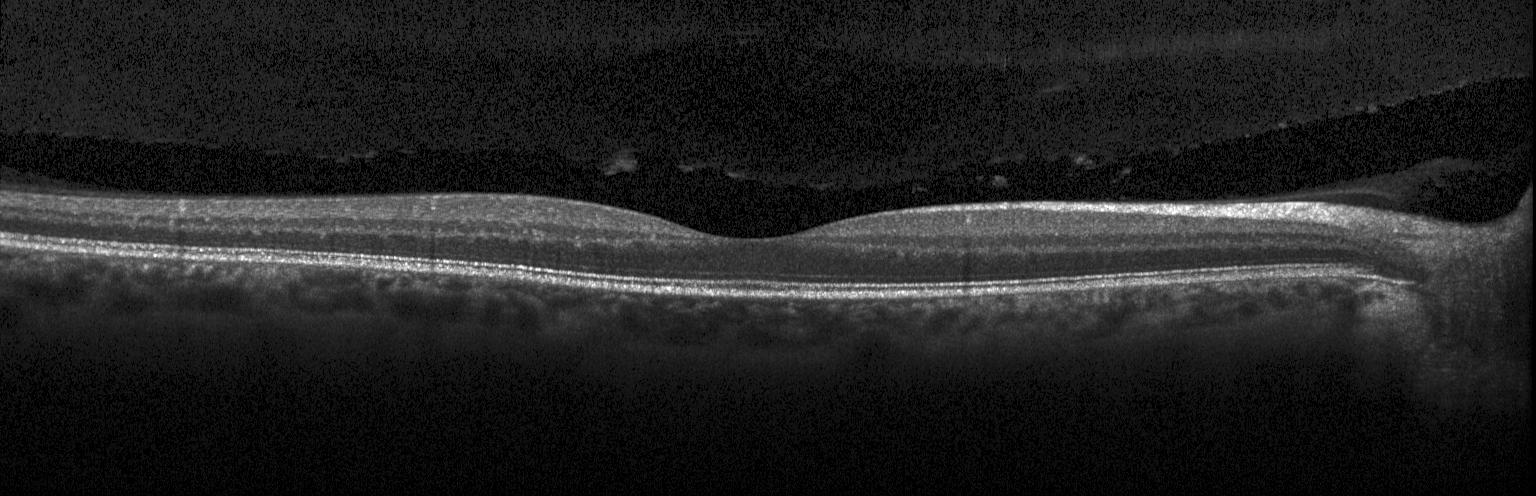

Through the macula, retinal OCT B-scan — The scan shows neither choroidal neovascularization, diabetic macular edema, nor drusen.